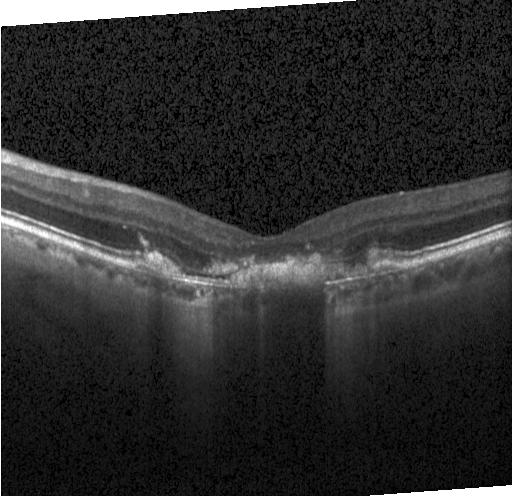
Finding: choroidal neovascularization.